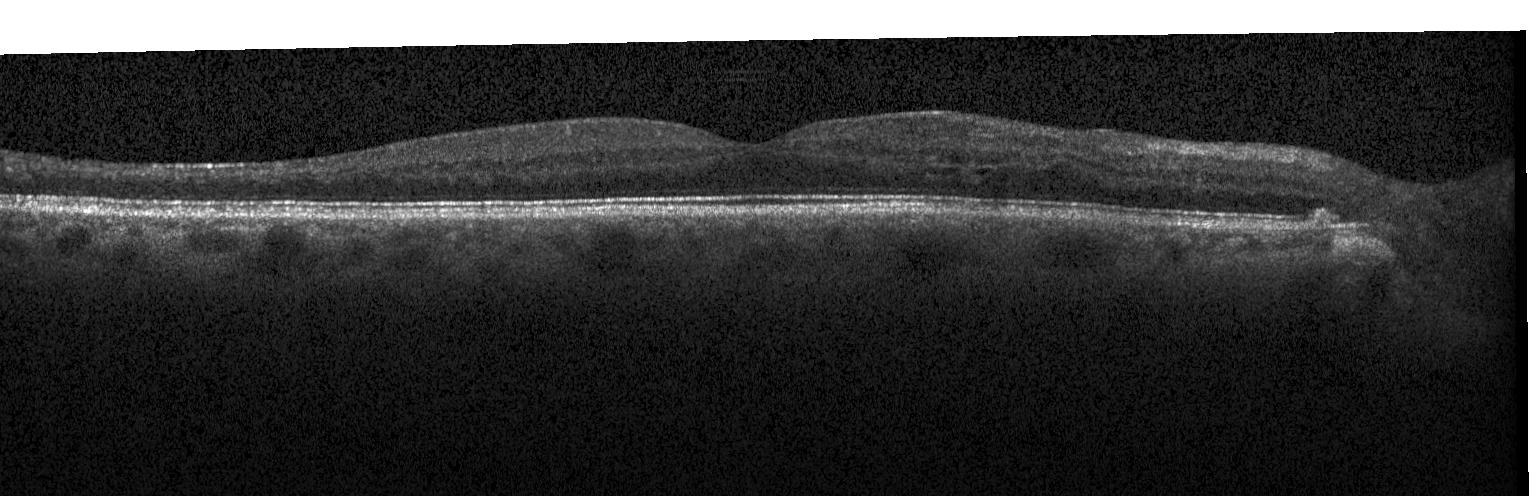
Impression: diabetic macular edema (DME).